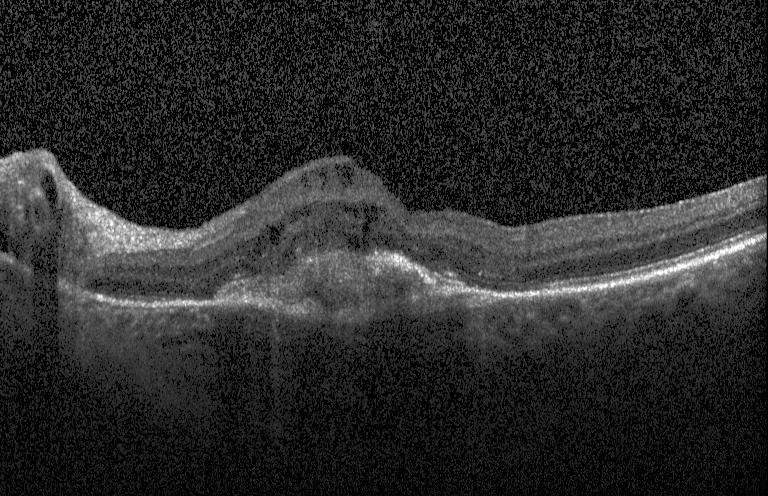 Macular OCT: choroidal neovascularization (CNV).